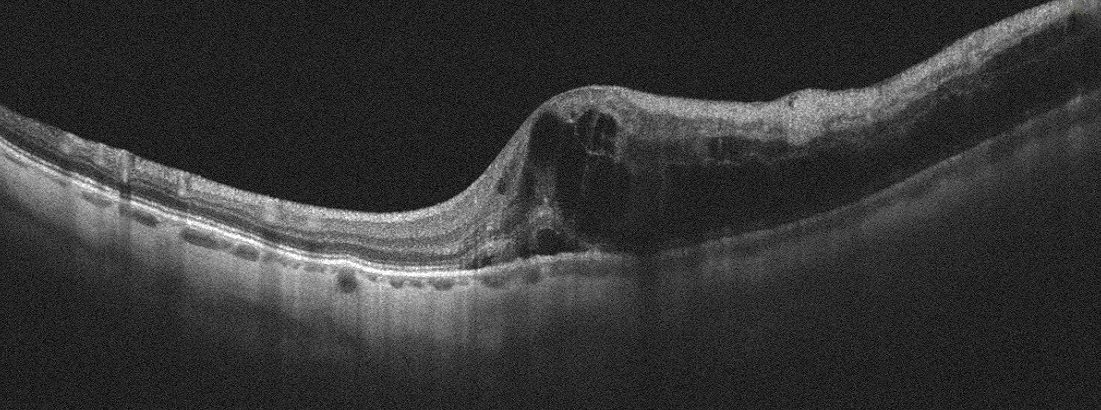

OCT B-scan, instrument: Optovue Avanti RTVue XR, macular scan — Assessment: retinal vein occlusion.